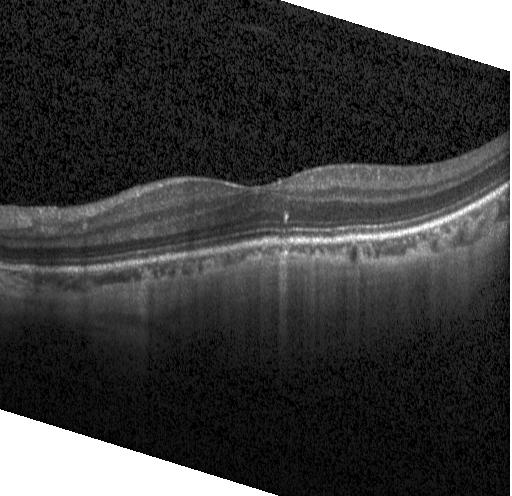 OCT scan showing no CNV, no DME, and no drusen.